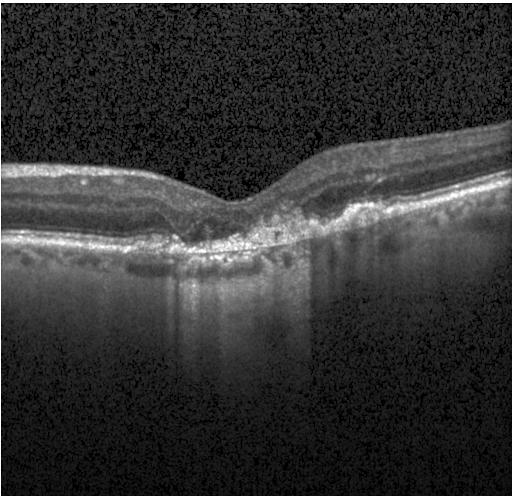
Diagnosis: a choroidal neovascular membrane.